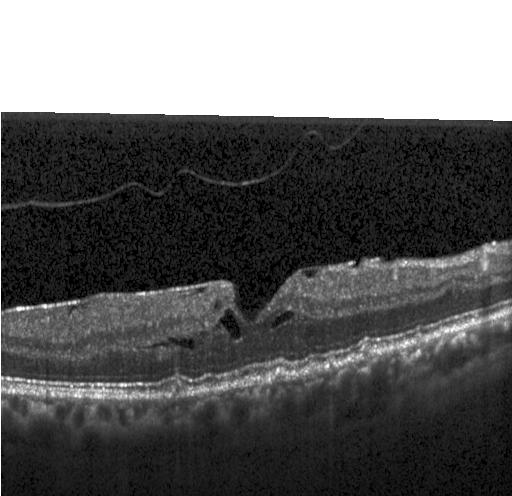

Instrument: Heidelberg Spectralis, spectral-domain OCT, OCT line scan, fovea-centered. Dx: multiple drusen.